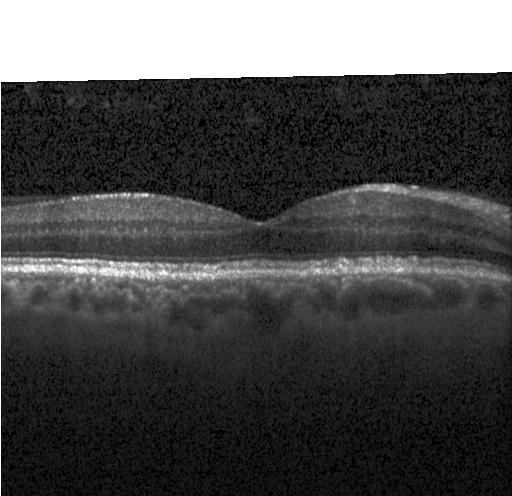

SD-OCT · retinal OCT cross-section. Assessment: no CNV, no DME, and no drusen.